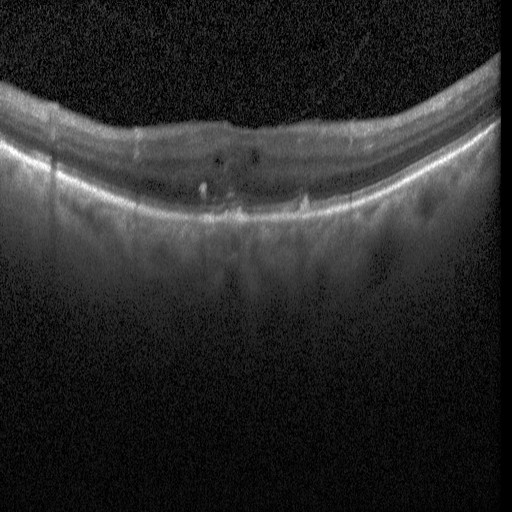
Optical coherence tomography scan
Assessment: DME.